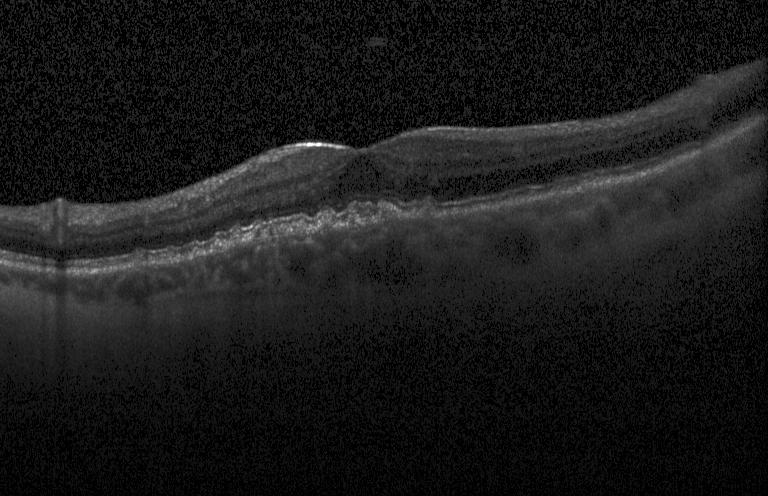
Retinal OCT cross-section showing drusen.